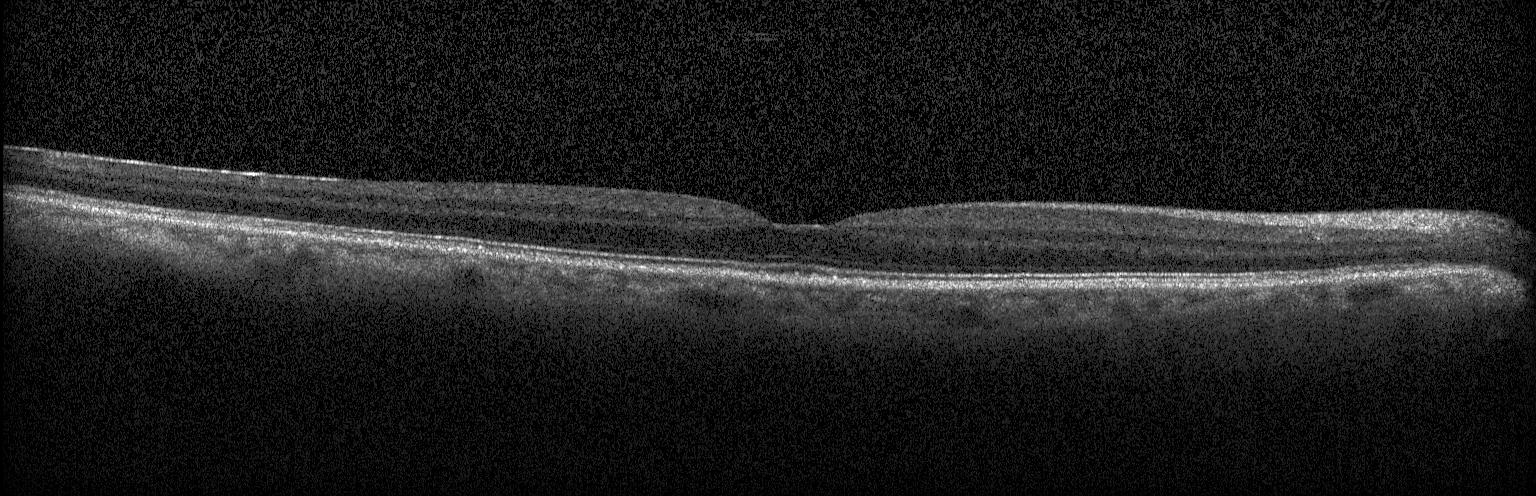
Finding: no CNV, DME, or drusen.